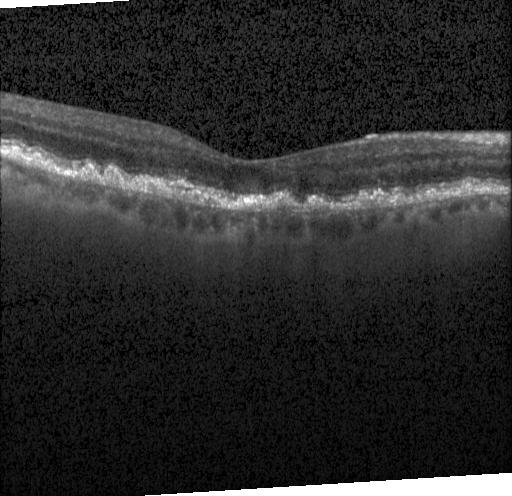

Optical coherence tomography scan · instrument: Heidelberg Spectralis. Assessment: choroidal neovascularization.